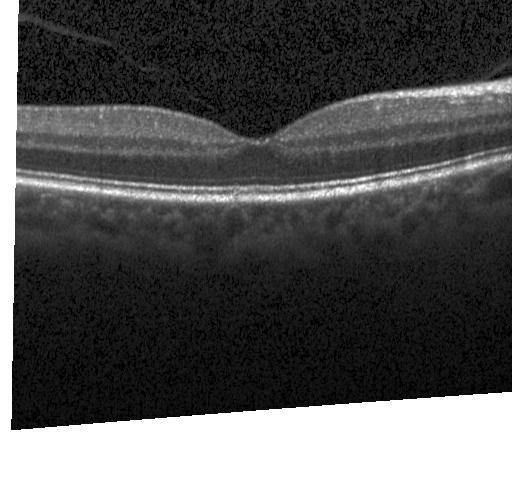
Optical coherence tomography scan. Macular scan. Spectral-domain OCT. Macular OCT: no choroidal neovascularization, diabetic macular edema, or drusen.